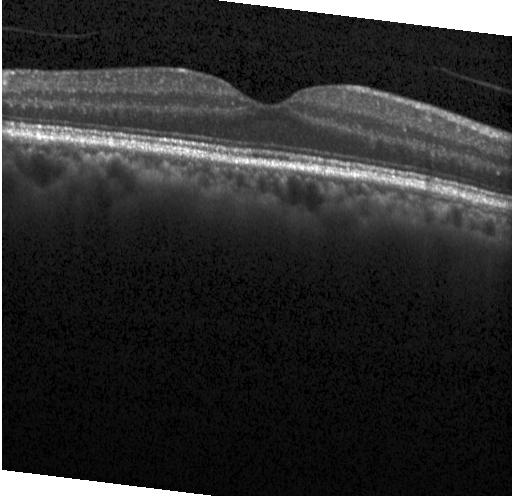

Spectral-domain OCT B-scan: neither choroidal neovascularization, diabetic macular edema, nor drusen.